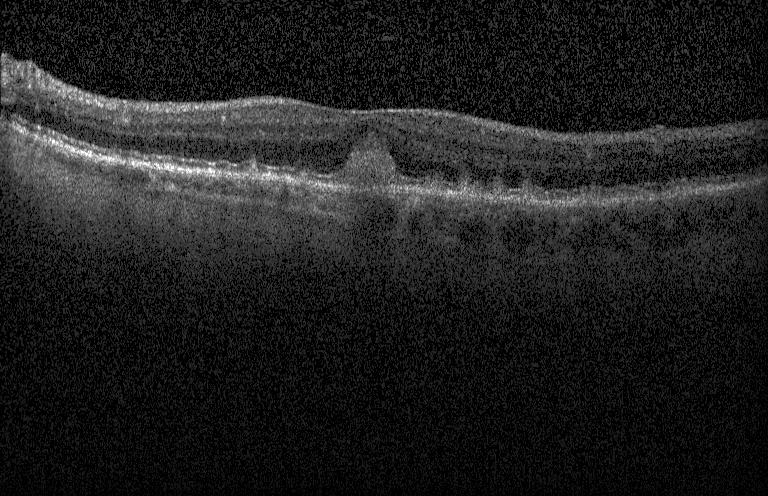

Diagnosis: a choroidal neovascular membrane.